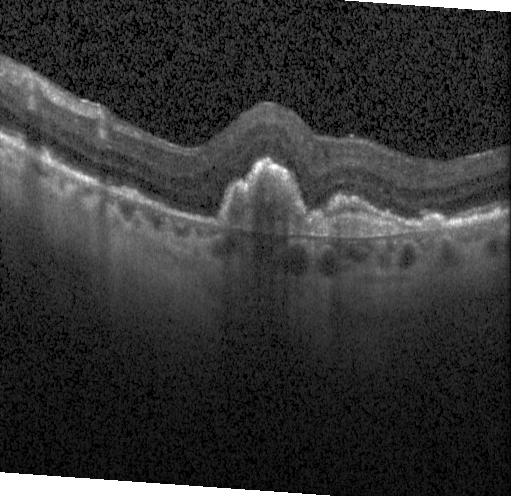
Acquired on a Heidelberg Spectralis, optical coherence tomography B-scan. The scan shows choroidal neovascularization (CNV).